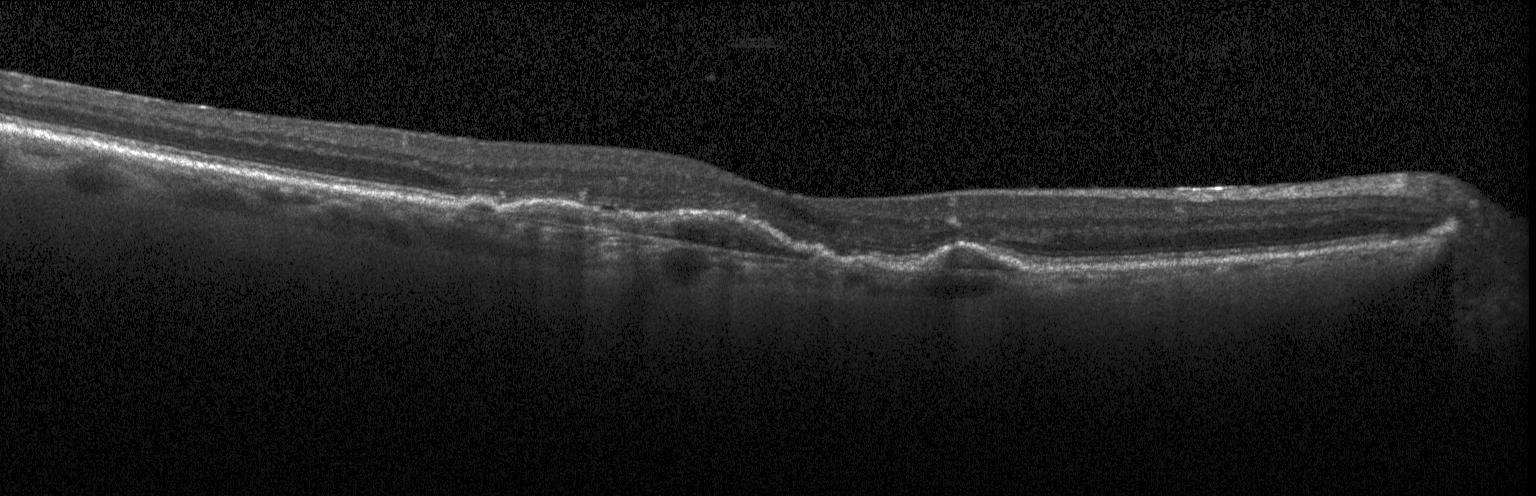 This B-scan demonstrates a choroidal neovascular membrane.